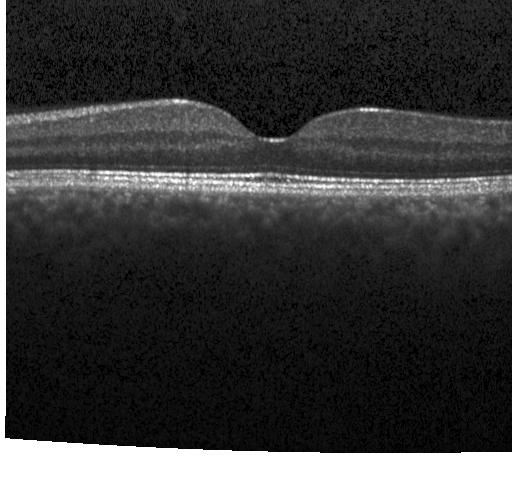 Optical coherence tomography B-scan, instrument: Heidelberg Spectralis, spectral-domain OCT. Dx: no evidence of CNV, DME, or drusen.